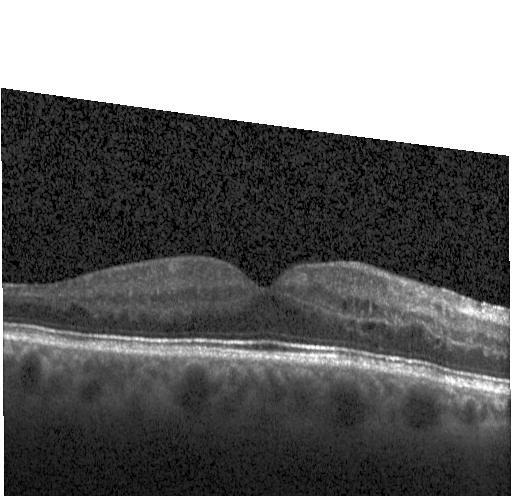
Impression: DME.